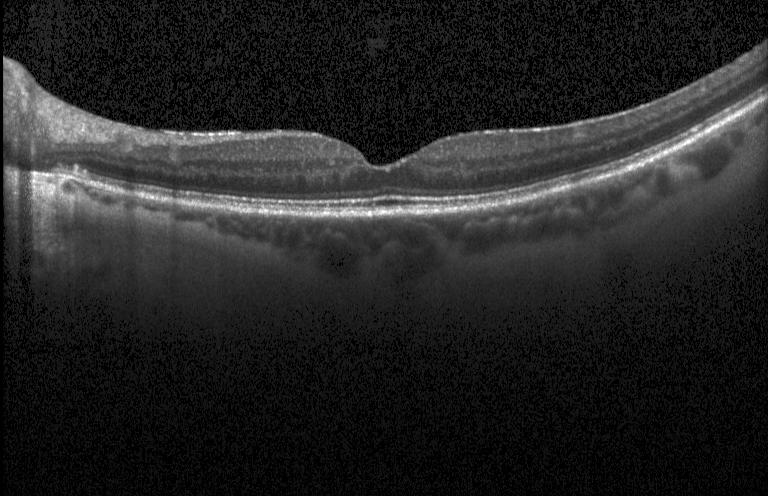 Instrument: Heidelberg Spectralis, retinal OCT B-scan, SD-OCT
Macular OCT: neither choroidal neovascularization, diabetic macular edema, nor drusen.